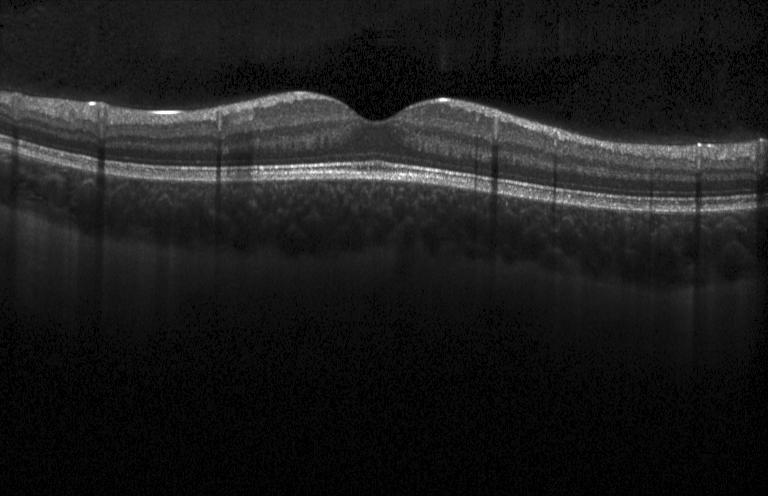
Centered on the fovea. SD-OCT. Optical coherence tomography B-scan. Heidelberg Spectralis OCT system
Macular OCT: neither choroidal neovascularization, diabetic macular edema, nor drusen.